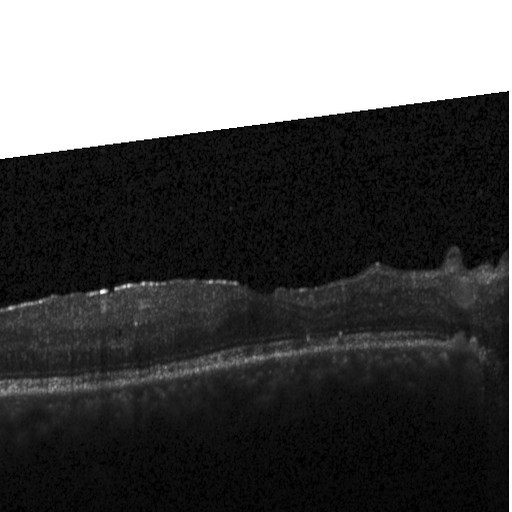
Through the macula, acquired on a Heidelberg Spectralis, optical coherence tomography scan, spectral-domain optical coherence tomography.
OCT finding: diabetic macular edema.